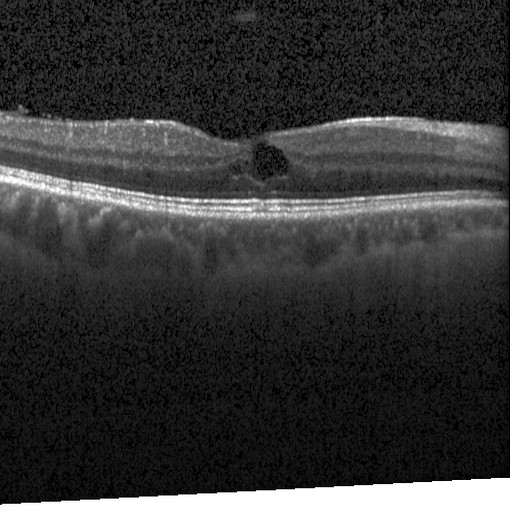 Diagnosis: diabetic macular edema (DME).